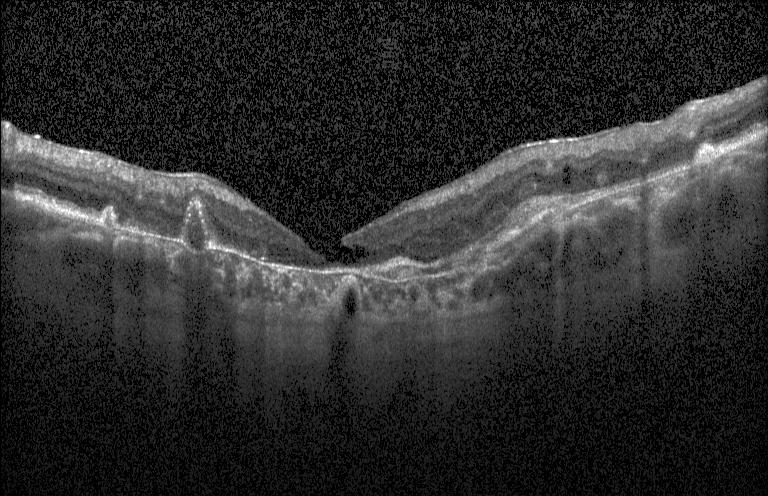

Fovea-centered, instrument: Heidelberg Spectralis, OCT line scan.
Assessment: choroidal neovascularization (CNV).